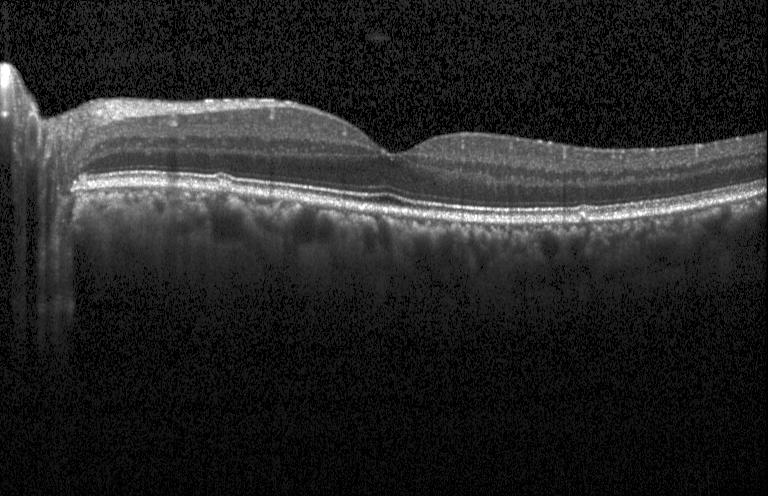 Retinal OCT B-scan; Heidelberg Spectralis OCT system; horizontal scan through the fovea — Sub-RPE drusenoid deposits.